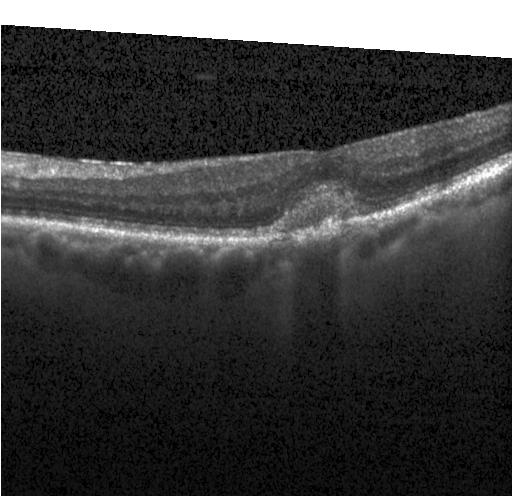
Impression: a choroidal neovascular membrane.